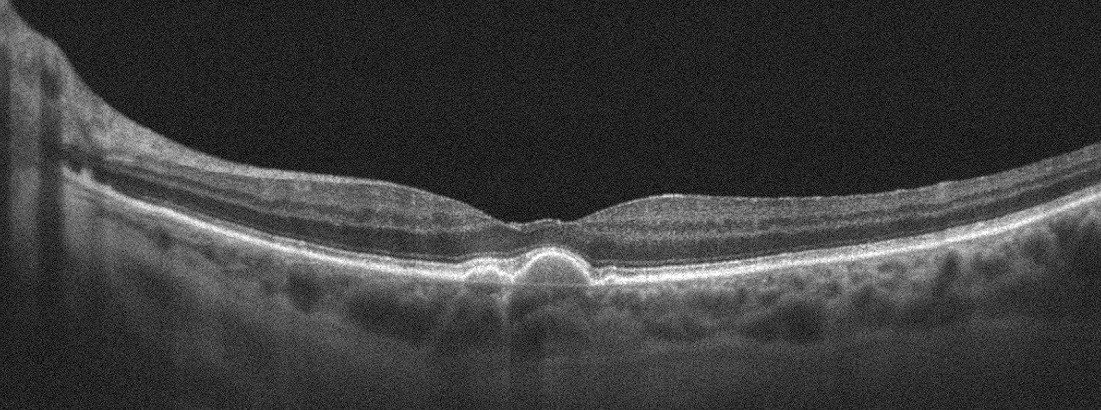 Diagnosis: AMD.